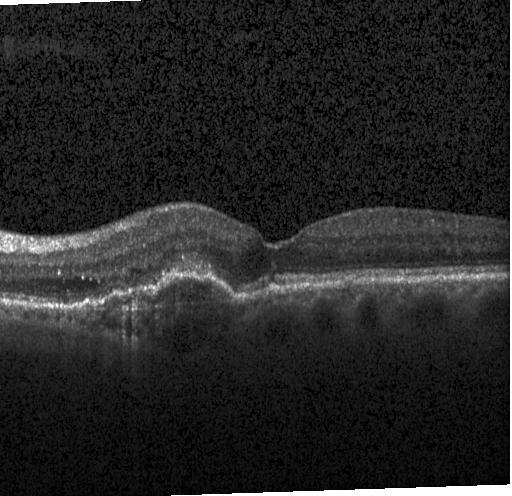
A choroidal neovascular membrane.